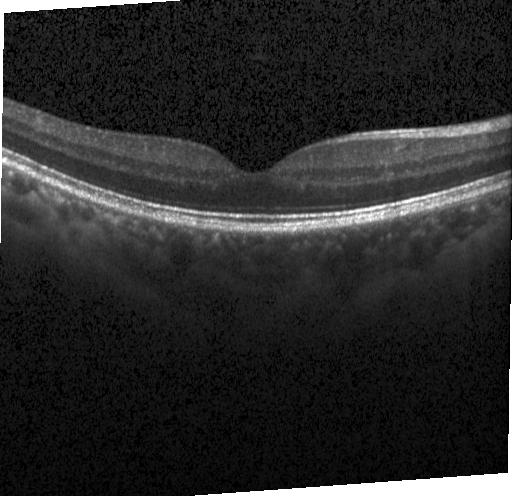
No choroidal neovascularization, no diabetic macular edema, and no drusen.